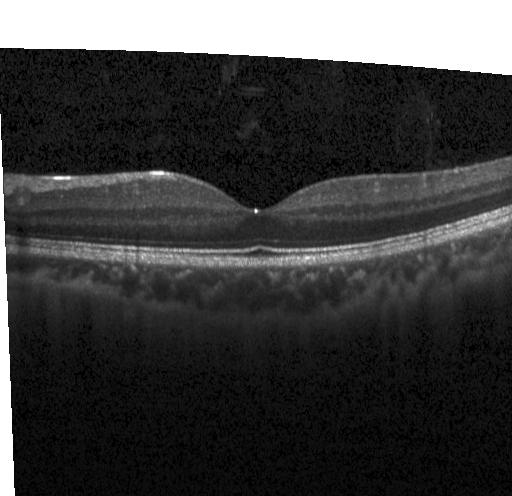

Finding: no CNV, no DME, and no drusen.